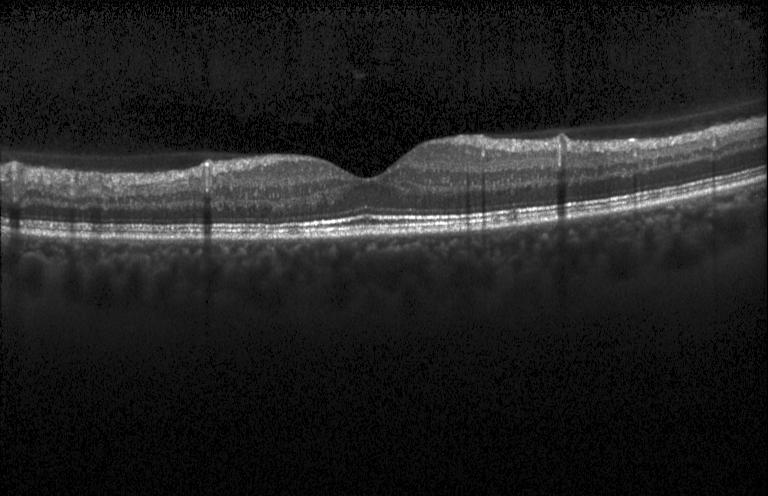

Optical coherence tomography B-scan
Impression: no evidence of choroidal neovascularization, diabetic macular edema, or drusen.